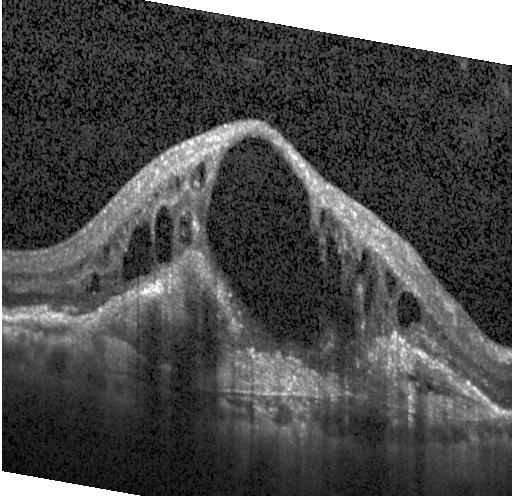 OCT line scan.
Diagnosis: choroidal neovascularization.